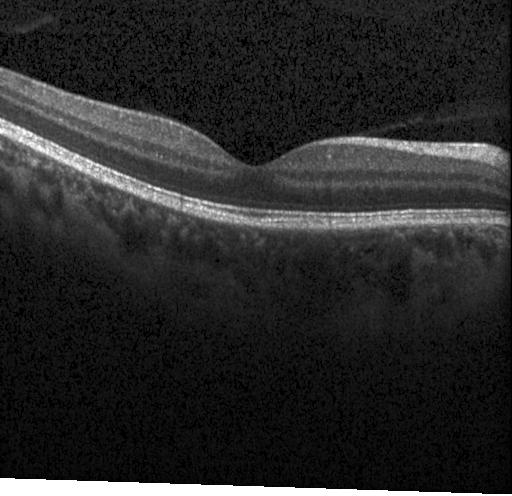
Finding: no choroidal neovascularization, no diabetic macular edema, and no drusen.